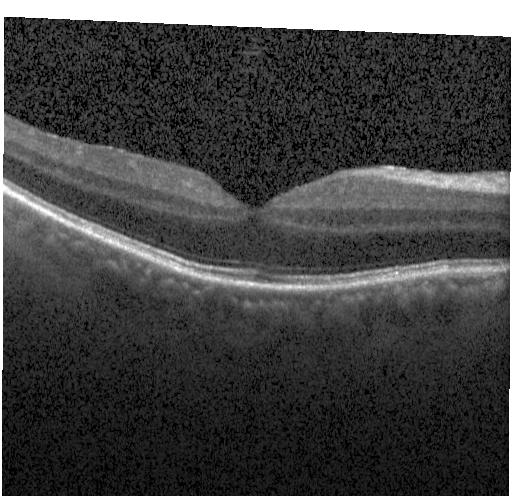
Macular OCT: no choroidal neovascularization, diabetic macular edema, or drusen.